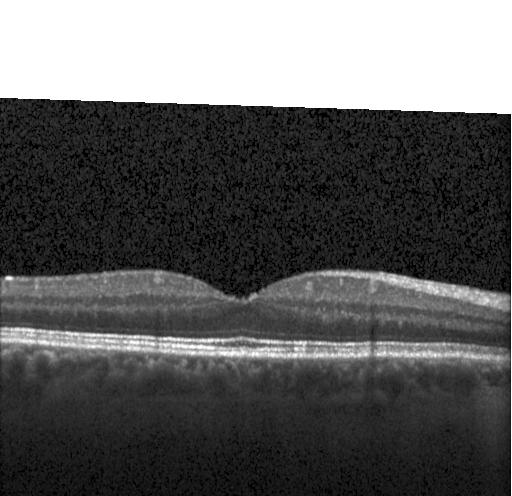

Macular OCT: no evidence of choroidal neovascularization, diabetic macular edema, or drusen.